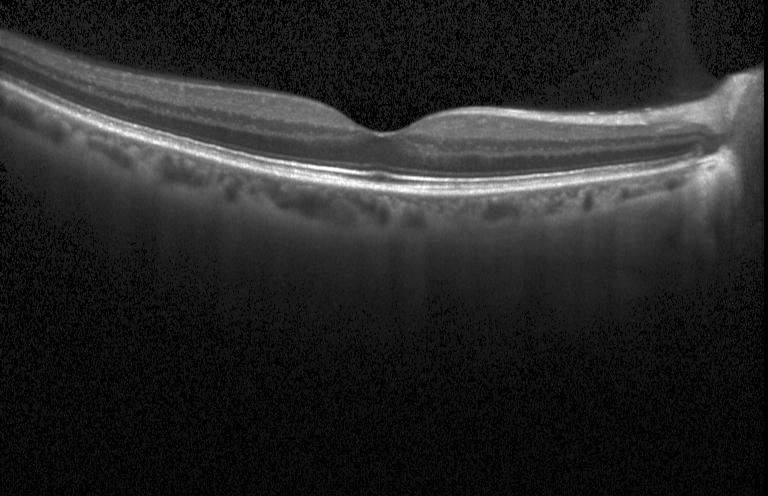
Heidelberg Spectralis. SD-OCT. OCT B-scan.
Impression: no CNV, DME, or drusen.